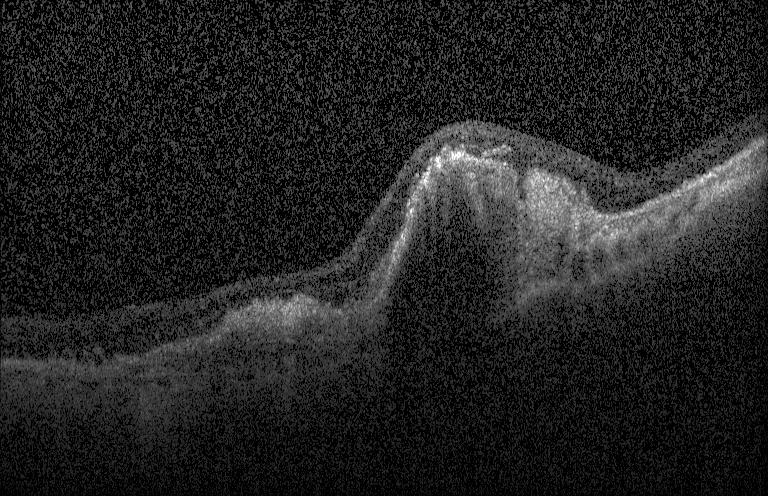

Instrument: Heidelberg Spectralis. Retinal OCT B-scan
This B-scan demonstrates choroidal neovascularization.